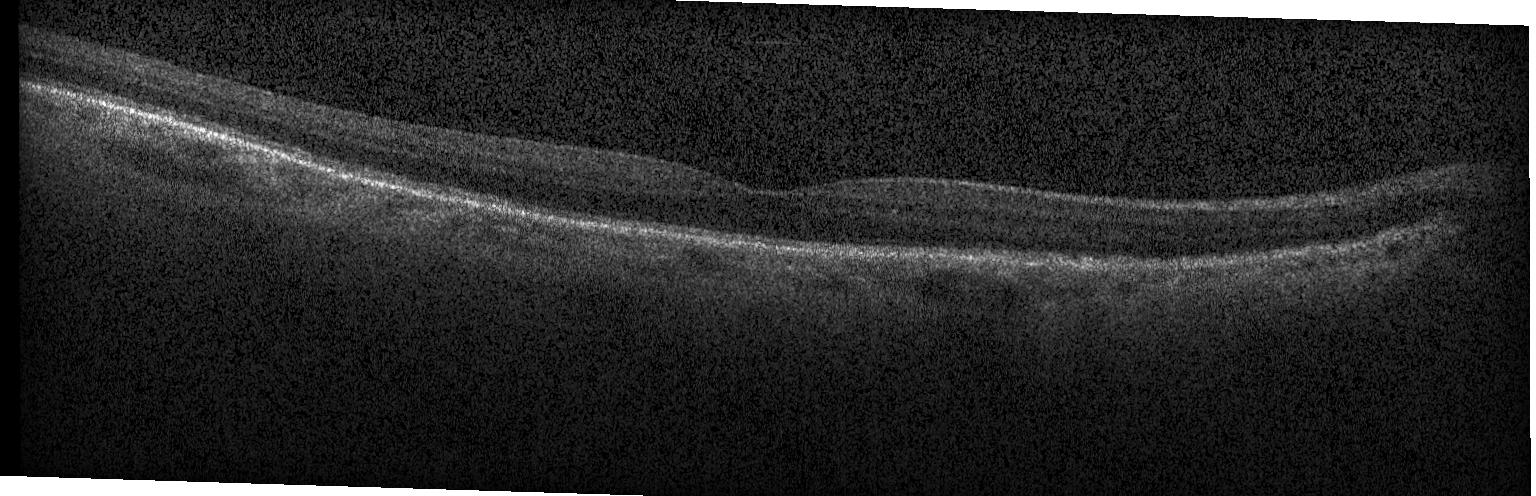 Retinal OCT cross-section showing neither CNV, DME, nor drusen.